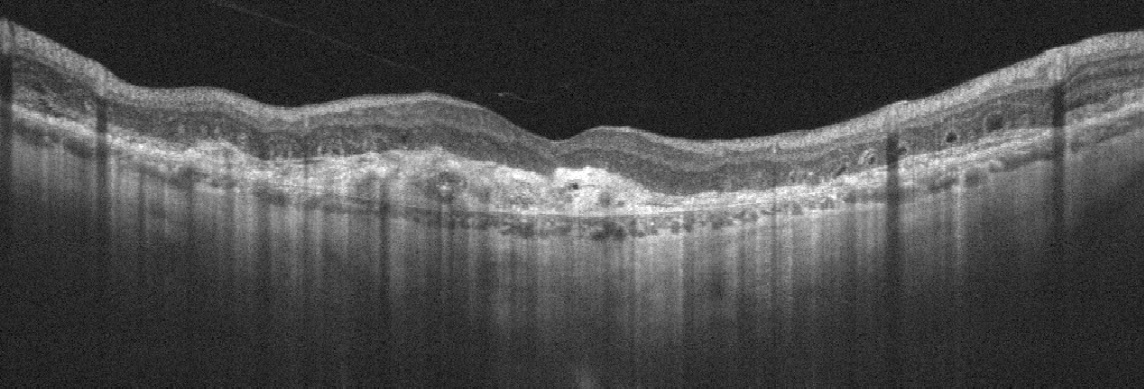
OCT scan showing AMD.